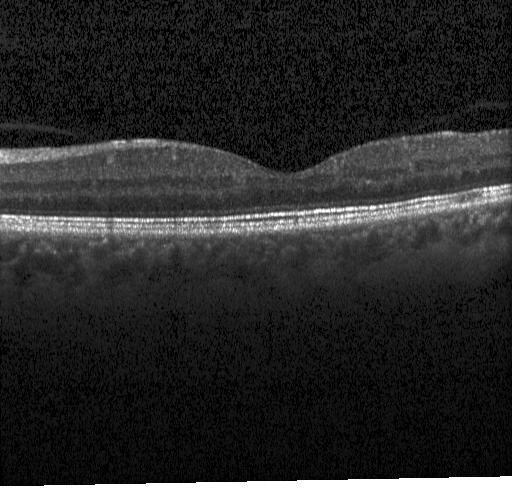
Impression: no CNV, no DME, and no drusen.